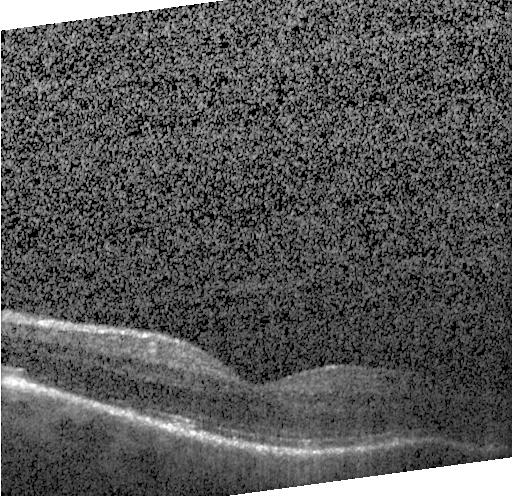 Spectral-domain OCT B-scan: no CNV, no DME, and no drusen.